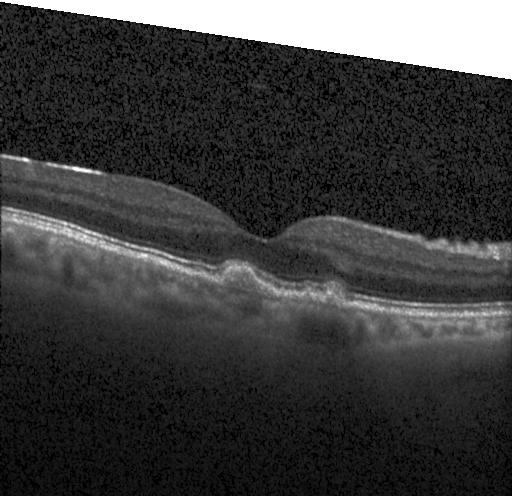

Acquired on a Heidelberg Spectralis · OCT B-scan. Finding: drusen.